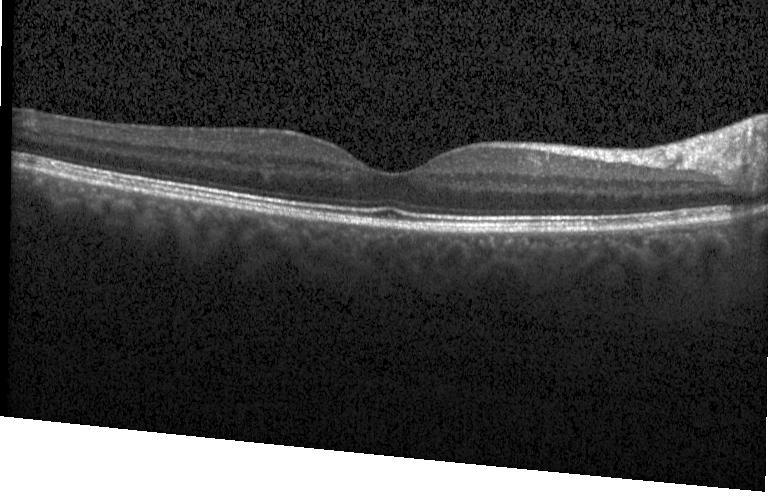
OCT scan showing no evidence of choroidal neovascularization, diabetic macular edema, or drusen.